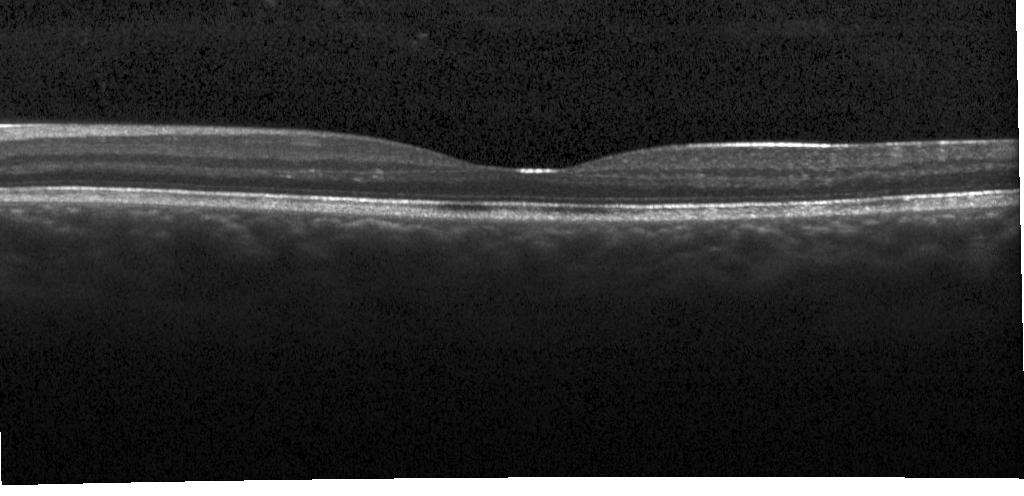

Optical coherence tomography scan, SD-OCT
The scan shows neither choroidal neovascularization, diabetic macular edema, nor drusen.